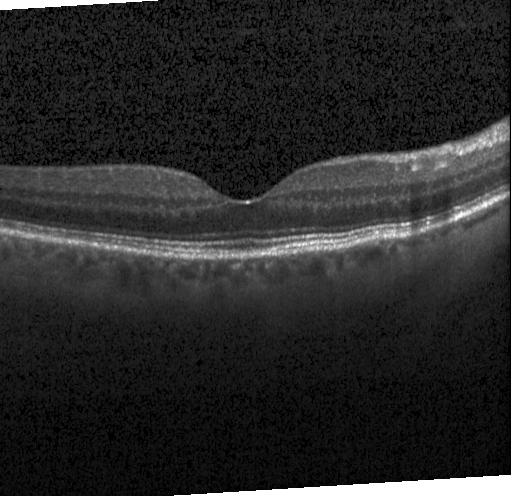 Dx: no evidence of choroidal neovascularization, diabetic macular edema, or drusen.